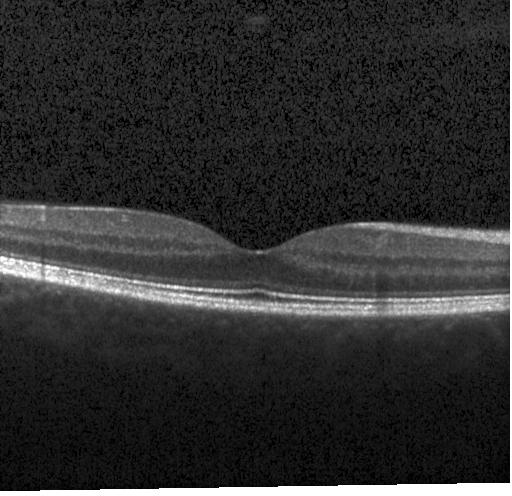 Diagnosis: no choroidal neovascularization, diabetic macular edema, or drusen.